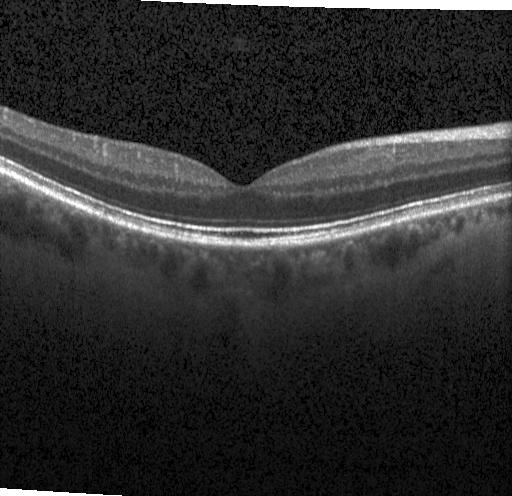
Heidelberg Spectralis; centered on the fovea; optical coherence tomography scan; spectral-domain optical coherence tomography — Assessment: no choroidal neovascularization, no diabetic macular edema, and no drusen.